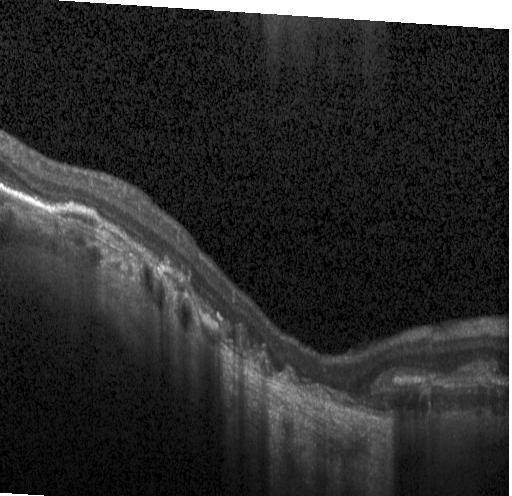
Retinal OCT cross-section showing a choroidal neovascular membrane.